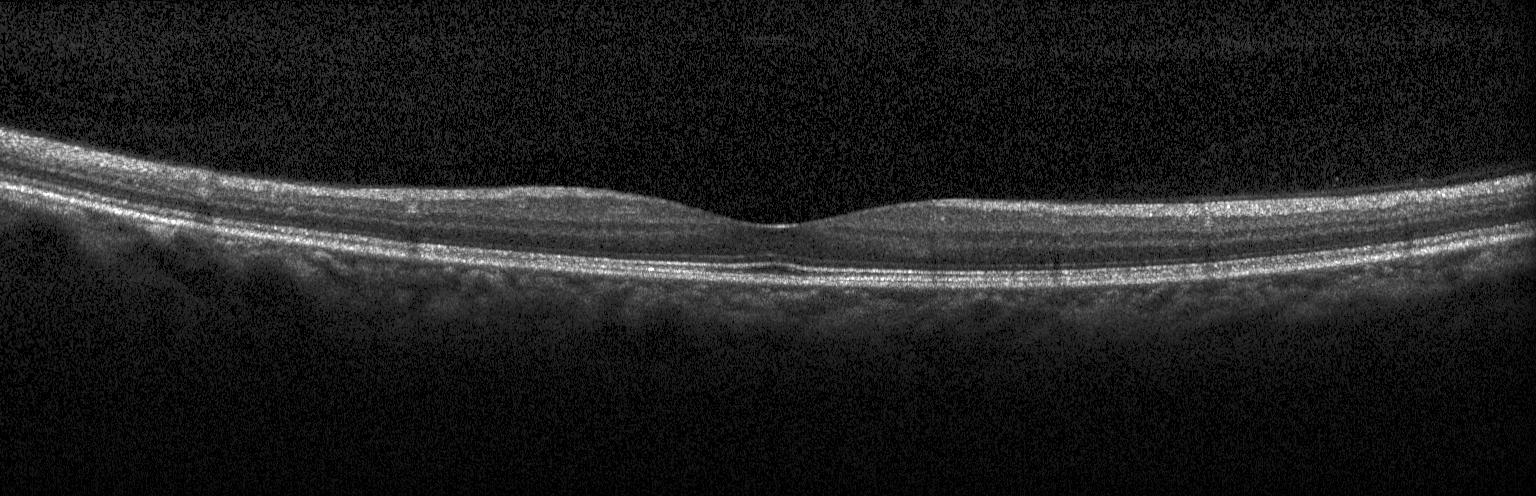

Instrument: Heidelberg Spectralis; spectral-domain OCT; optical coherence tomography B-scan. No choroidal neovascularization, no diabetic macular edema, and no drusen.